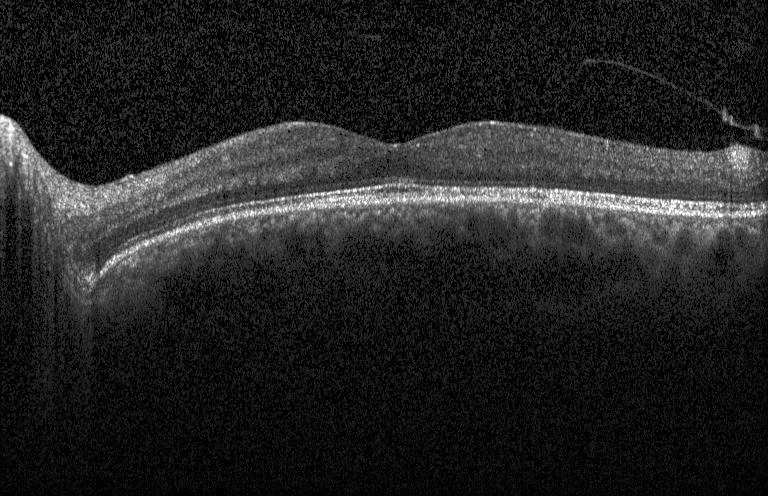
Assessment: no CNV, DME, or drusen.